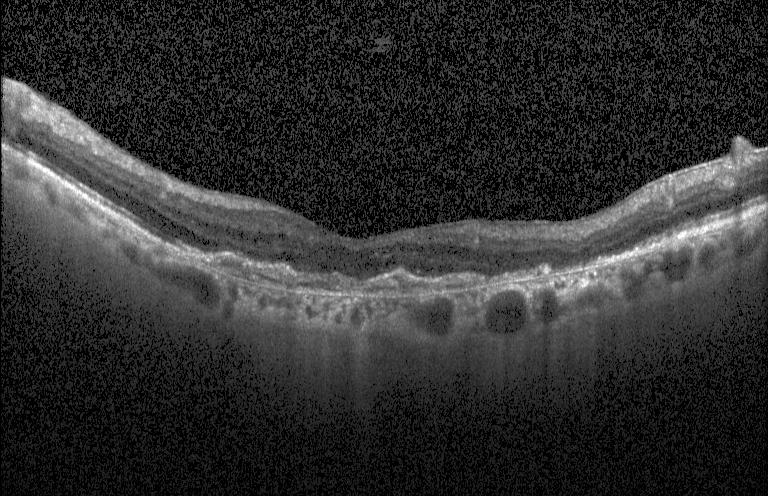

Heidelberg Spectralis OCT system; optical coherence tomography scan. Diagnosis: a choroidal neovascular membrane.